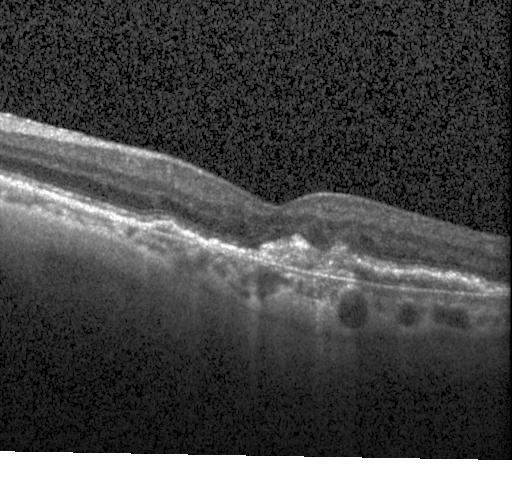 Optical coherence tomography B-scan, Heidelberg Spectralis, horizontal scan through the fovea, SD-OCT. Finding: choroidal neovascularization.